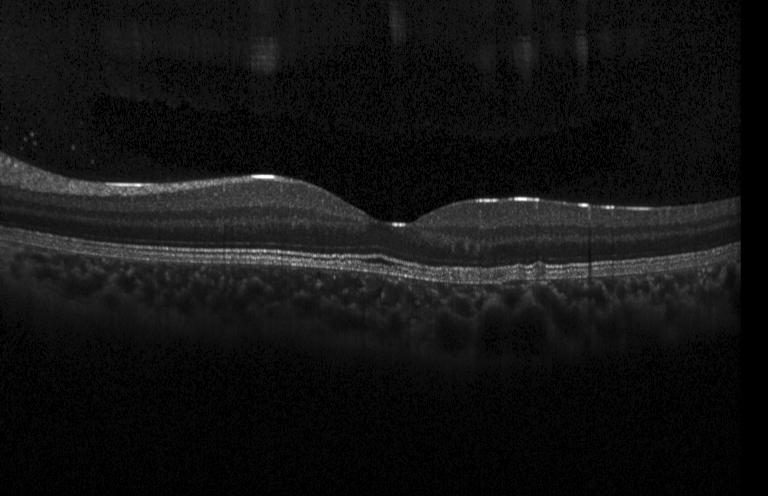 SD-OCT · Heidelberg Spectralis OCT system · through the macula · optical coherence tomography B-scan — This B-scan demonstrates no choroidal neovascularization, no diabetic macular edema, and no drusen.